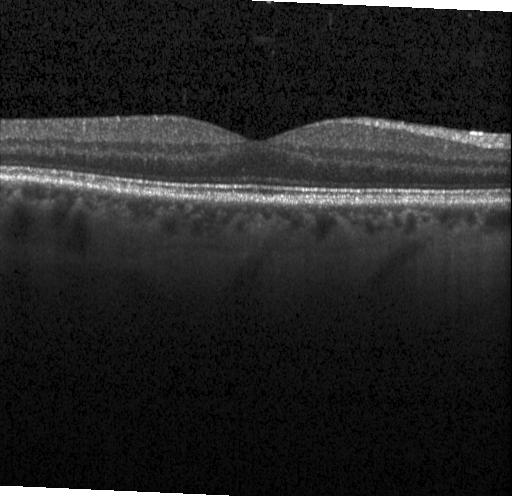
OCT line scan. Acquired on a Heidelberg Spectralis. Fovea-centered.
Finding: no choroidal neovascularization, diabetic macular edema, or drusen.